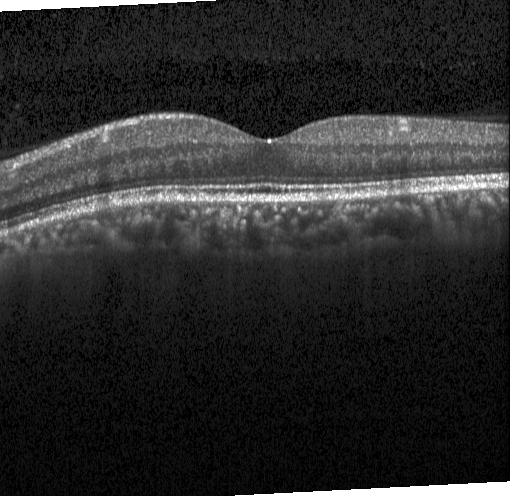
Spectral-domain OCT. Optical coherence tomography B-scan. Through the macula. Heidelberg Spectralis.
Impression: no choroidal neovascularization, diabetic macular edema, or drusen.